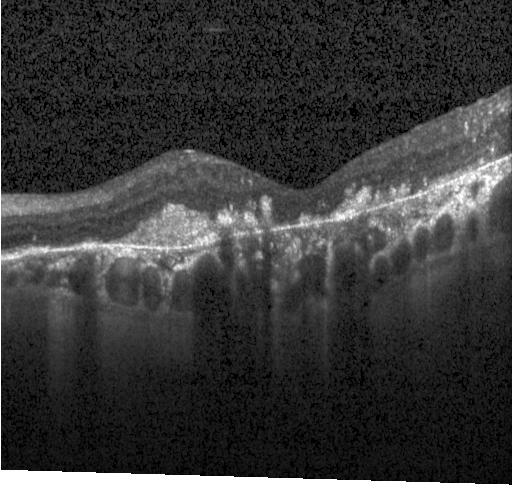 OCT B-scan showing choroidal neovascularization.